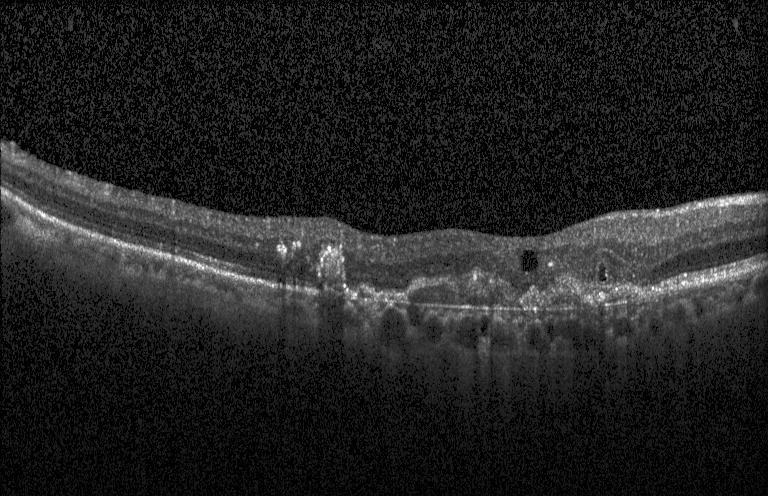

Instrument: Heidelberg Spectralis · OCT B-scan — Diagnosis: choroidal neovascularization (CNV).